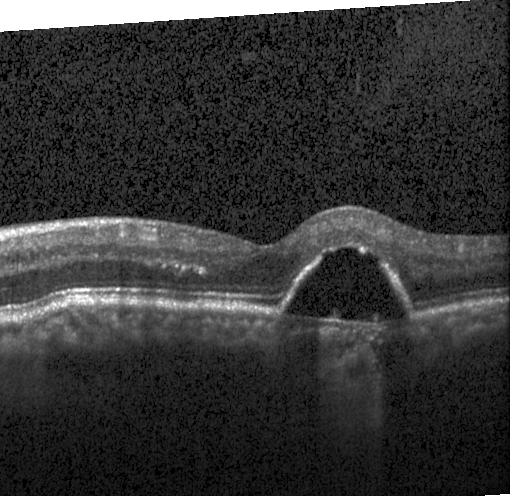

Diagnosis: a choroidal neovascular membrane.